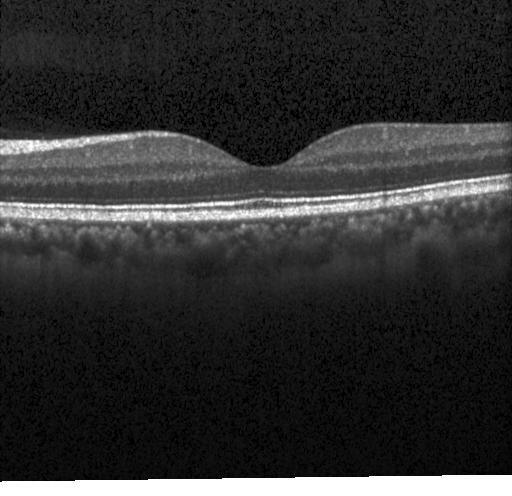 Macular OCT demonstrating neither choroidal neovascularization, diabetic macular edema, nor drusen.